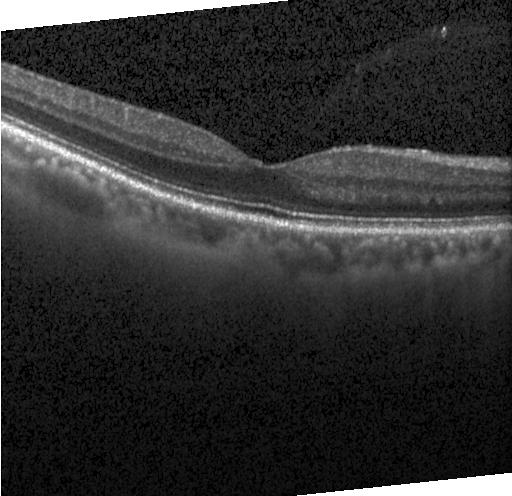

Finding: no CNV, no DME, and no drusen.